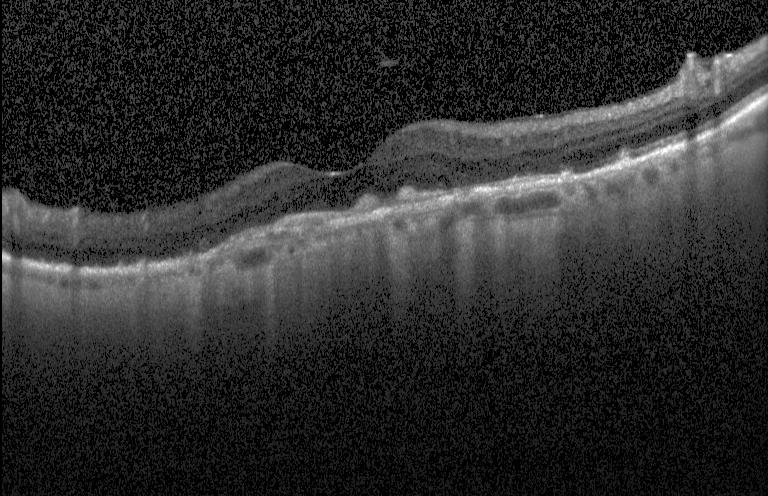

Centered on the fovea, spectral-domain OCT, retinal OCT B-scan.
Impression: choroidal neovascularization.